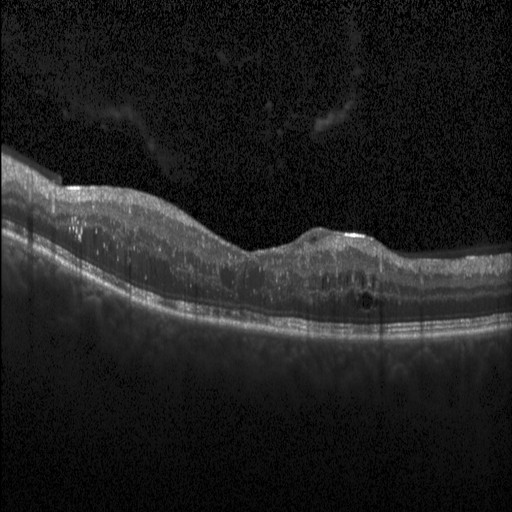

Optical coherence tomography B-scan, horizontal scan through the fovea — Finding: diabetic macular edema.